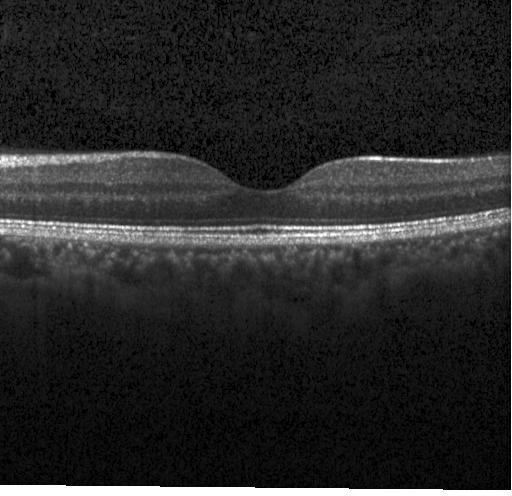

Fovea-centered · retinal OCT B-scan.
Impression: neither choroidal neovascularization, diabetic macular edema, nor drusen.